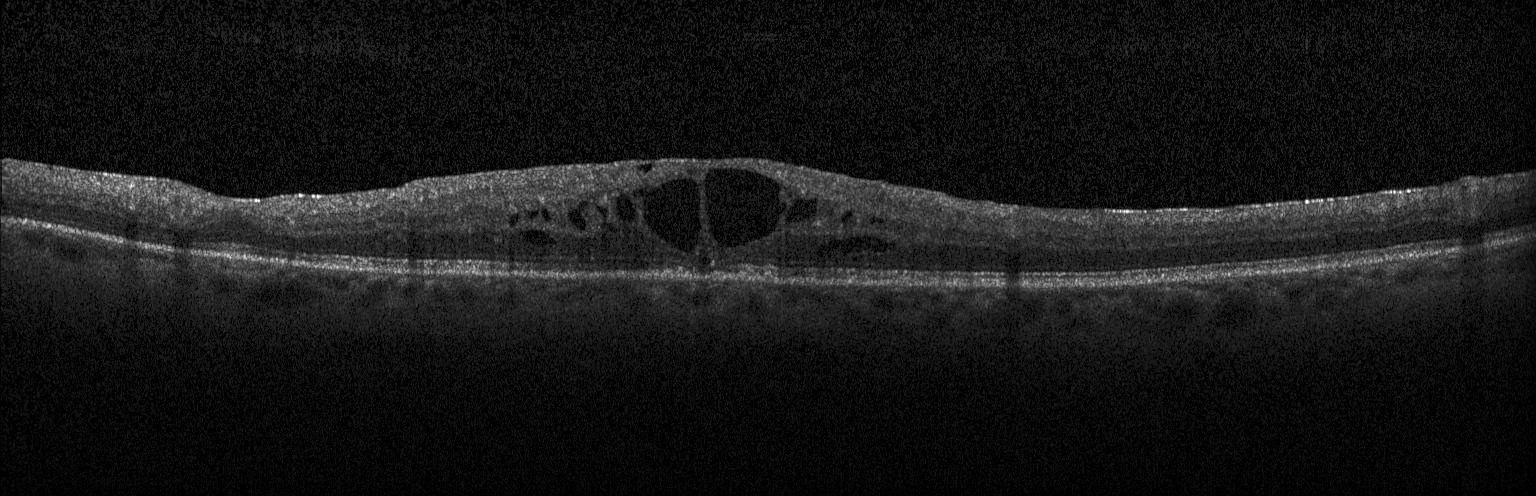
OCT B-scan, Heidelberg Spectralis OCT system, spectral-domain OCT
Diagnosis: diabetic macular edema (DME).